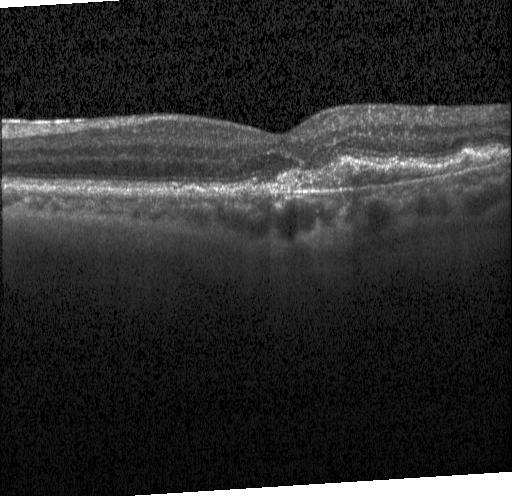

Spectral-domain OCT; instrument: Heidelberg Spectralis; retinal OCT cross-section; horizontal scan through the fovea — This B-scan demonstrates a choroidal neovascular membrane.